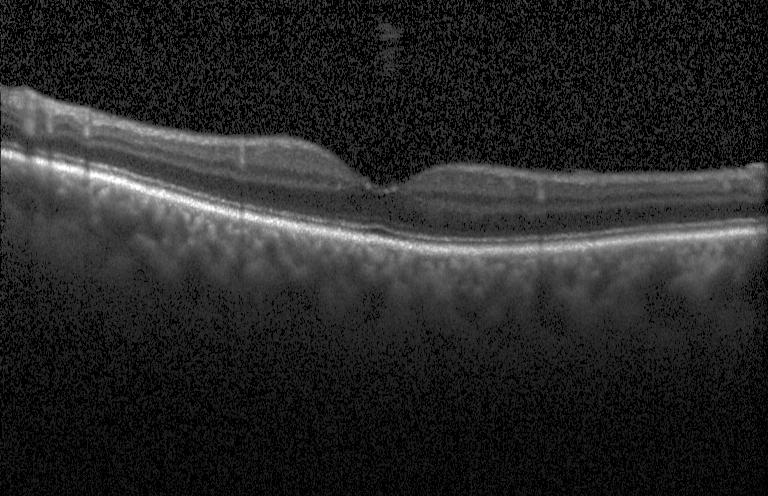

Retinal OCT B-scan — Assessment: neither choroidal neovascularization, diabetic macular edema, nor drusen.